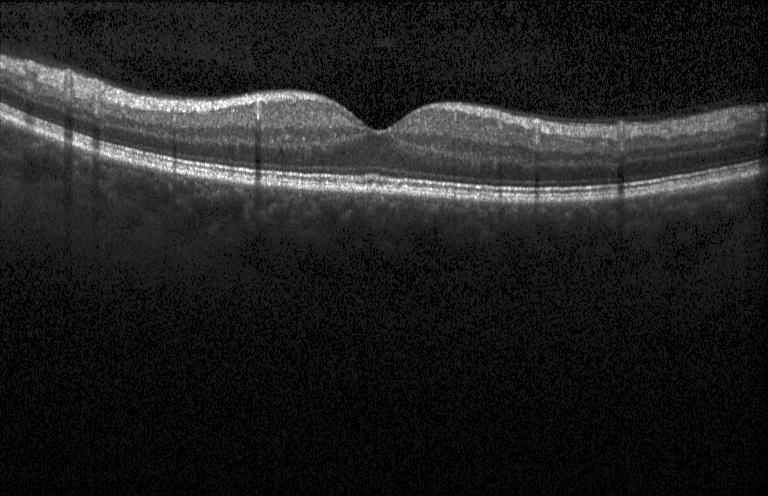
Macular scan. Retinal OCT cross-section. SD-OCT. Heidelberg Spectralis.
Dx: neither CNV, DME, nor drusen.